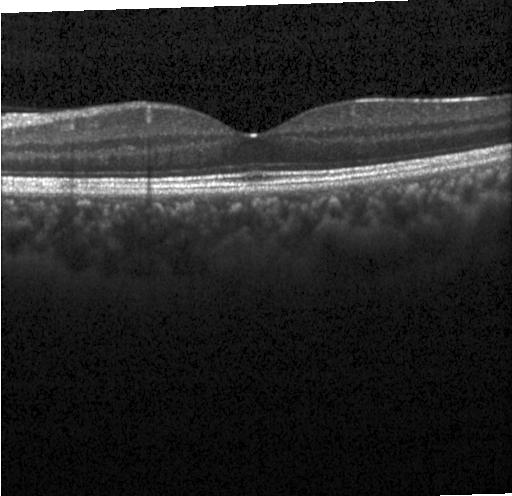

Centered on the fovea · optical coherence tomography scan
Impression: no choroidal neovascularization, diabetic macular edema, or drusen.